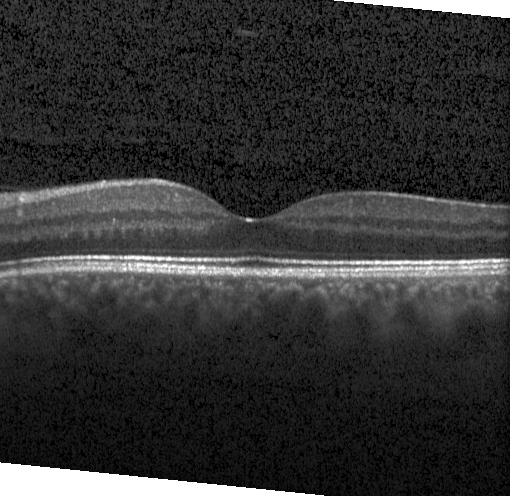
Macular OCT: no CNV, DME, or drusen.